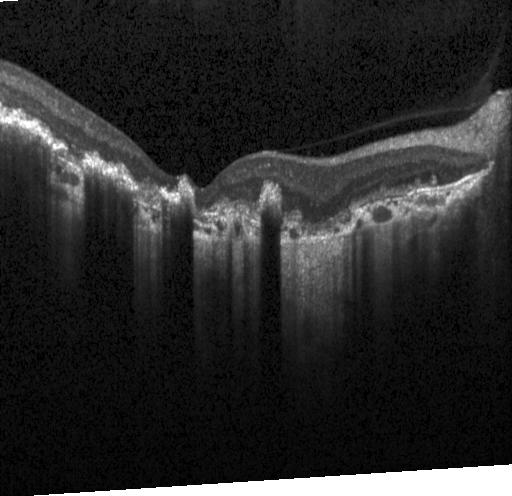

Spectral-domain OCT B-scan: a choroidal neovascular membrane.